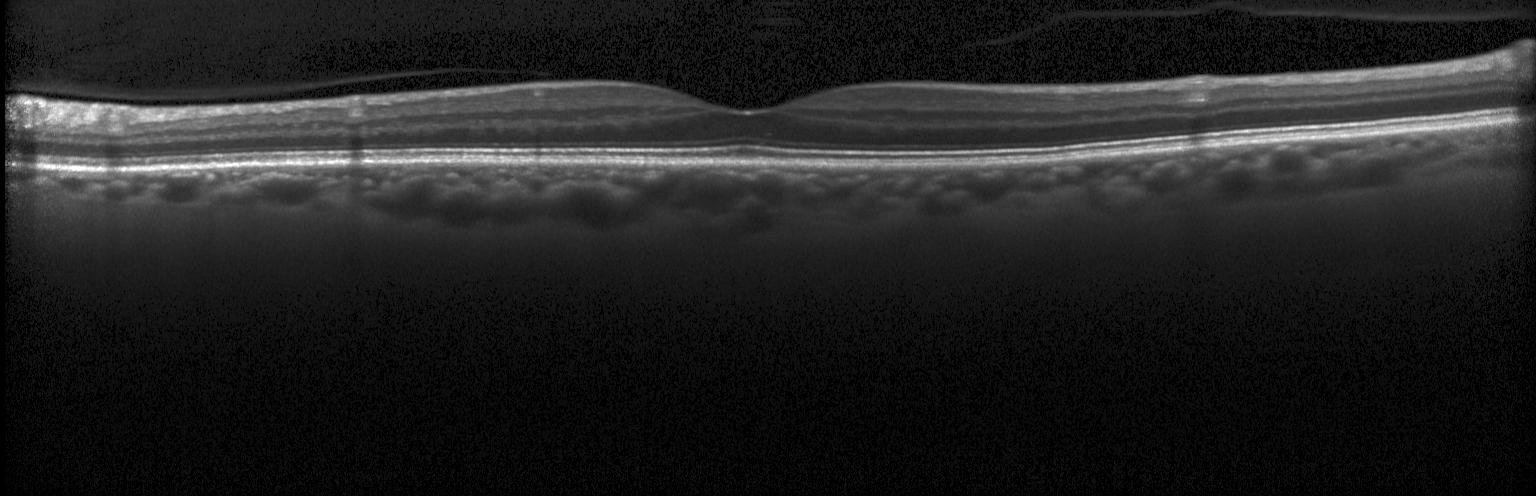
Centered on the fovea, retinal OCT B-scan.
Assessment: no CNV, no DME, and no drusen.